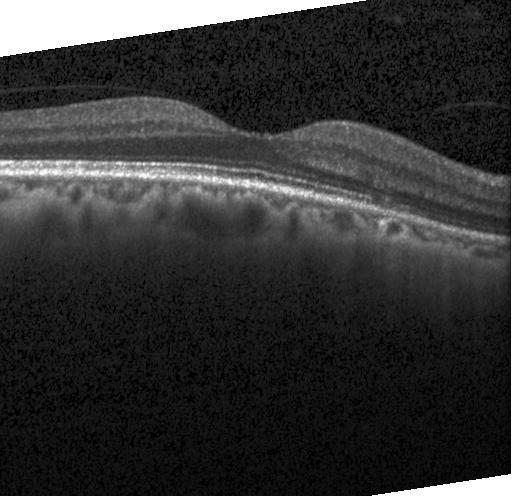
OCT line scan. Neither choroidal neovascularization, diabetic macular edema, nor drusen.